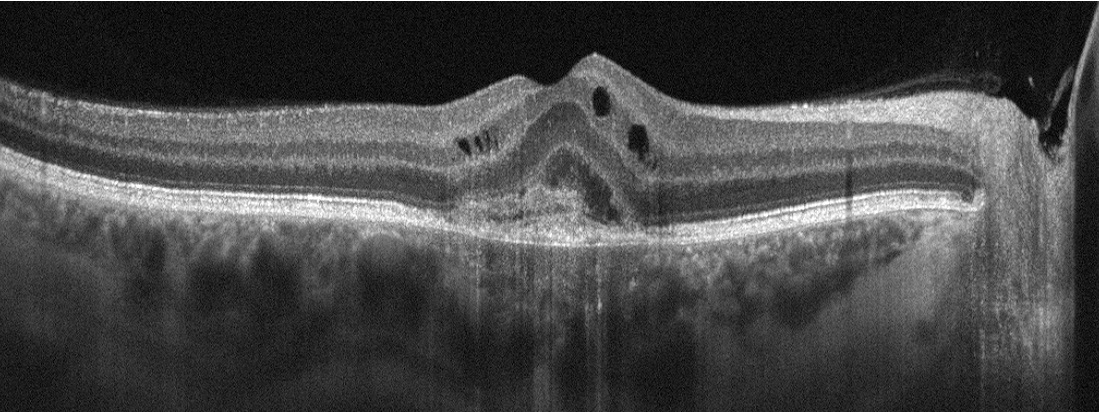 Finding: age-related macular degeneration.